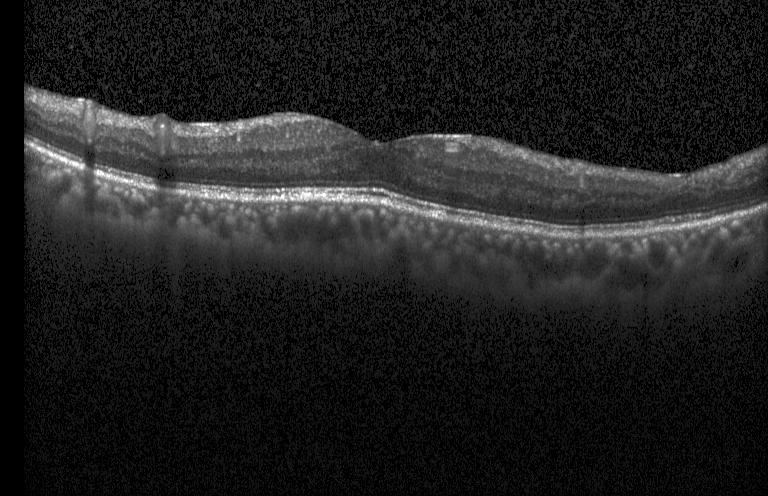

Dx: no evidence of choroidal neovascularization, diabetic macular edema, or drusen.